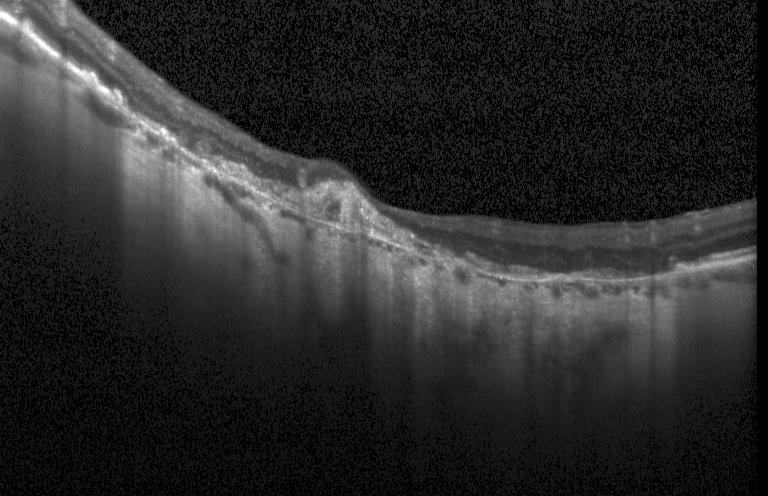

Instrument: Heidelberg Spectralis. Optical coherence tomography scan. Fovea-centered — Impression: a choroidal neovascular membrane.